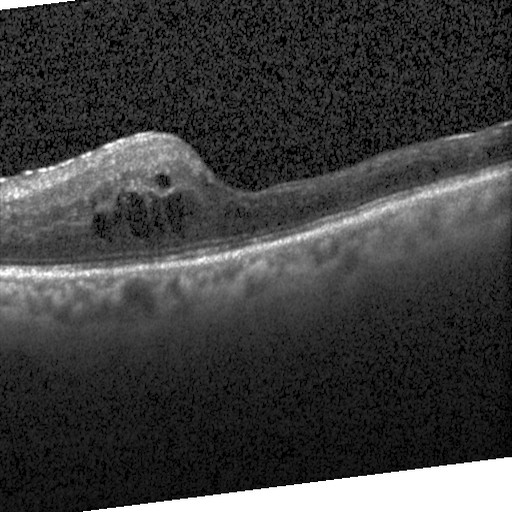
Fovea-centered. OCT B-scan
The scan shows diabetic macular edema (DME).